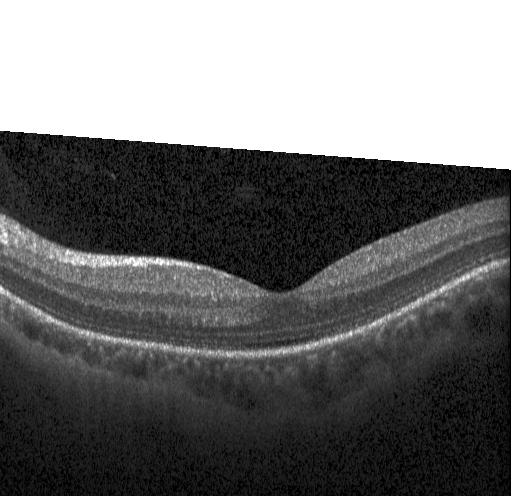

SD-OCT. Horizontal scan through the fovea. Heidelberg Spectralis OCT system. Retinal OCT B-scan. This B-scan demonstrates neither CNV, DME, nor drusen.